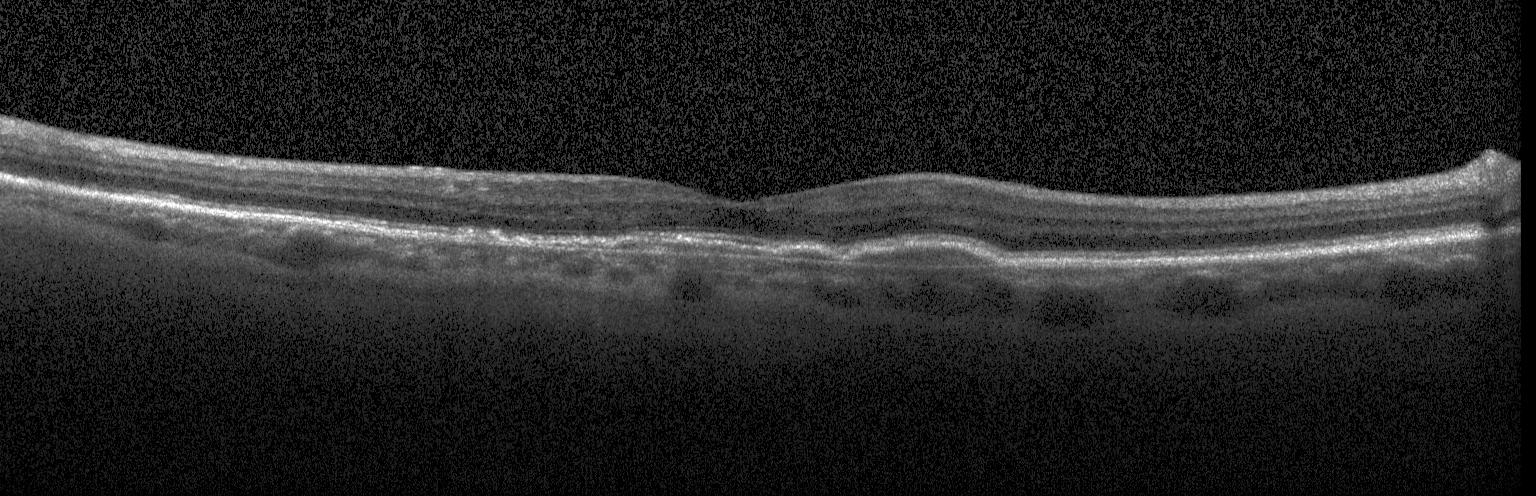

Assessment: a choroidal neovascular membrane.